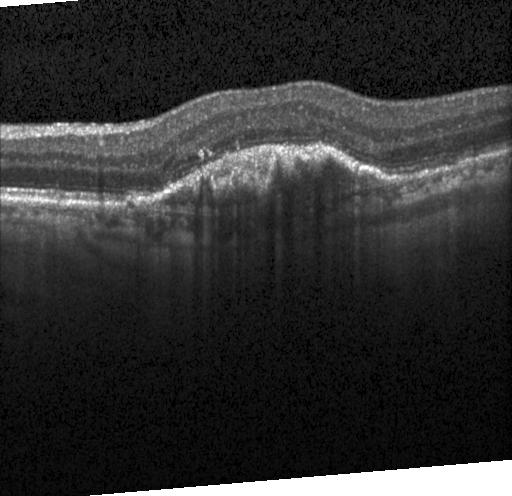

Optical coherence tomography B-scan.
A choroidal neovascular membrane.